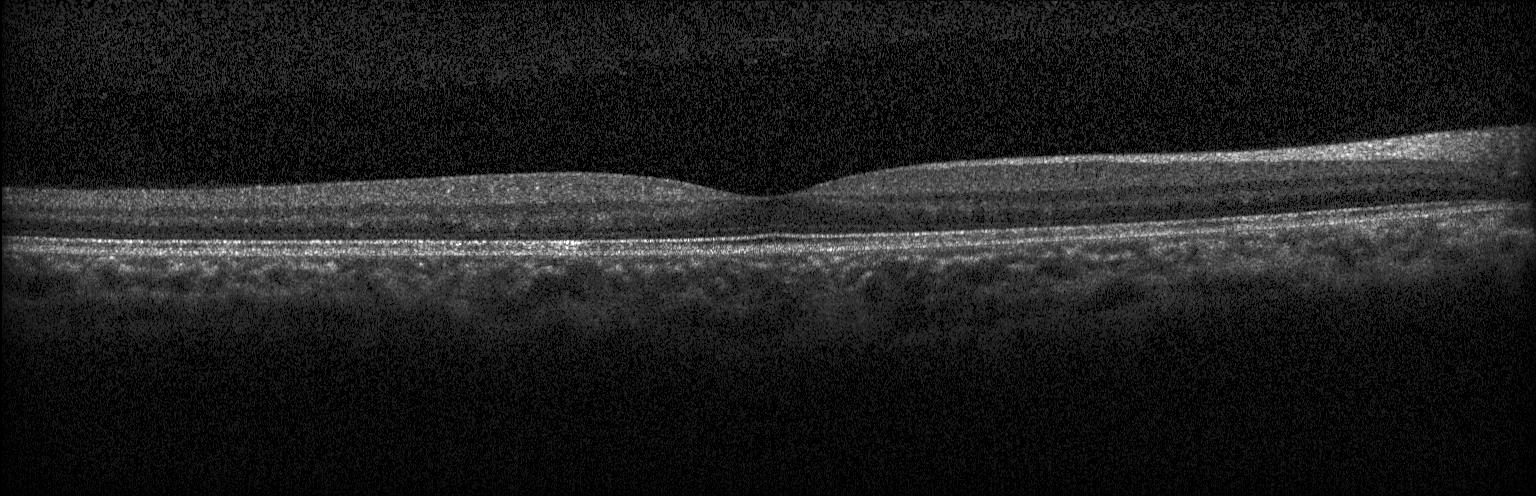

OCT line scan.
Finding: no evidence of choroidal neovascularization, diabetic macular edema, or drusen.